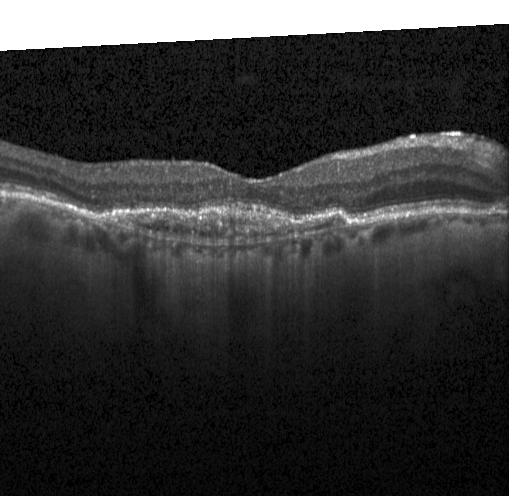 Optical coherence tomography scan. Spectral-domain OCT. Centered on the fovea
Macular OCT: CNV.